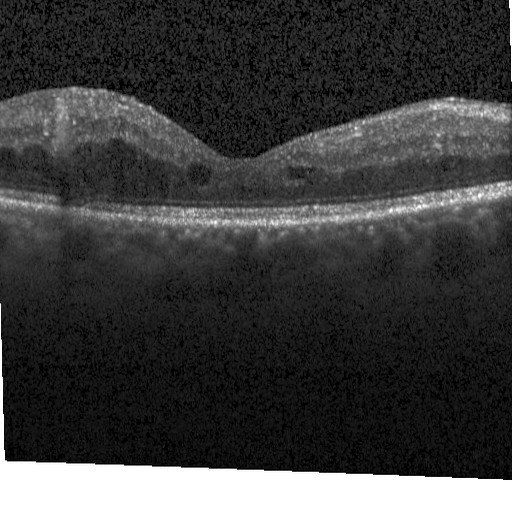 Diagnosis: diabetic macular edema (DME).